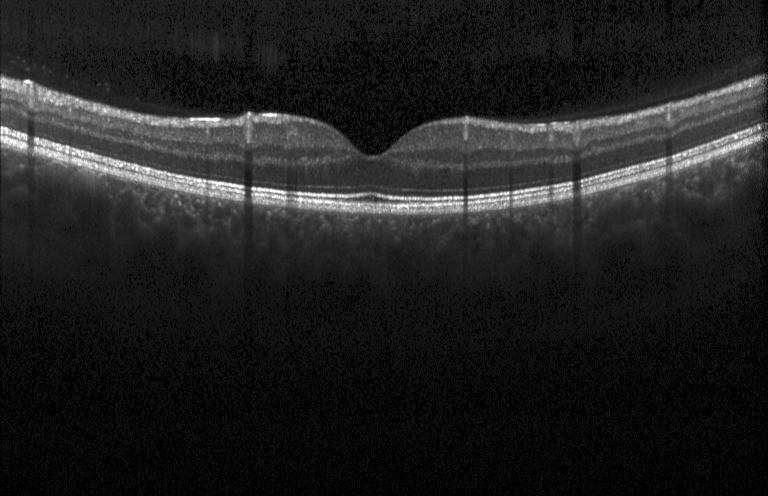

Horizontal scan through the fovea · OCT B-scan · Heidelberg Spectralis.
Macular OCT: neither choroidal neovascularization, diabetic macular edema, nor drusen.